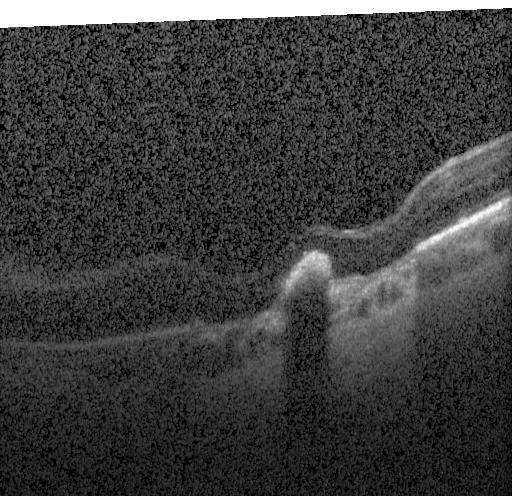
Fovea-centered · optical coherence tomography B-scan. This B-scan demonstrates a choroidal neovascular membrane.